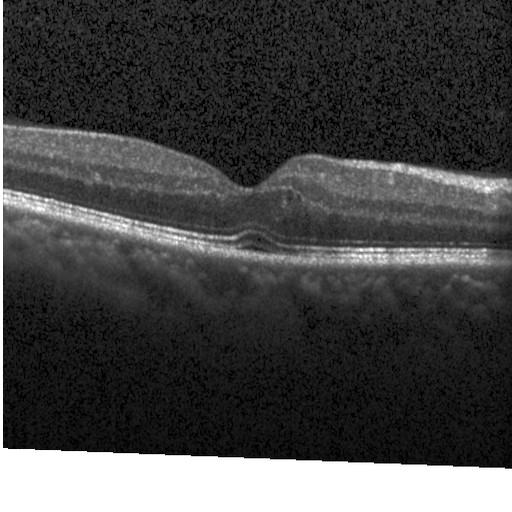
Finding: diabetic macular edema.